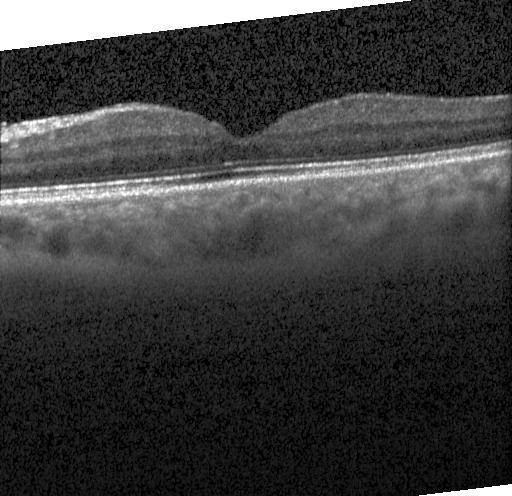

OCT line scan.
Neither CNV, DME, nor drusen.